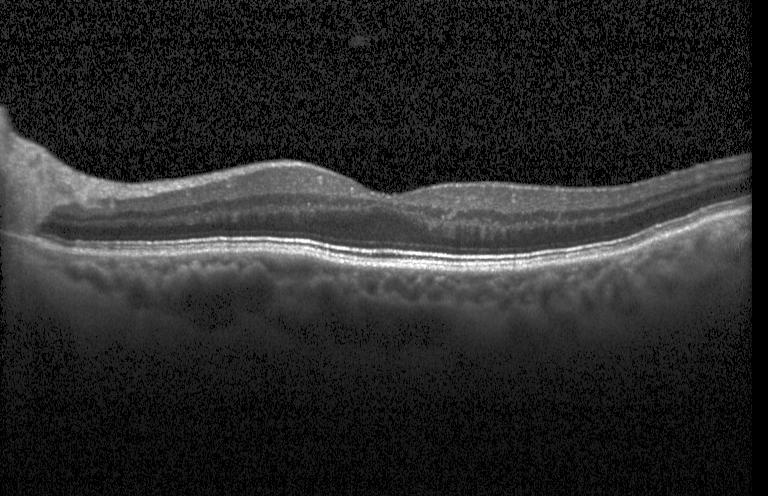 Horizontal scan through the fovea; instrument: Heidelberg Spectralis; retinal OCT B-scan. This B-scan demonstrates no evidence of CNV, DME, or drusen.